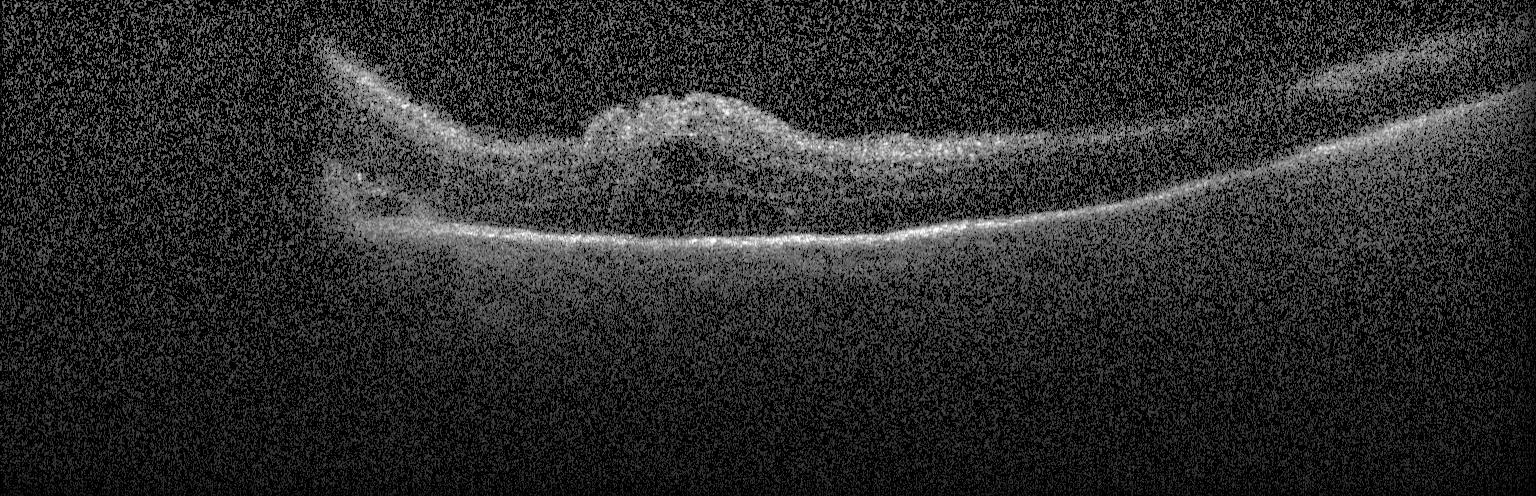 Spectral-domain OCT. Optical coherence tomography scan. Fovea-centered. Diabetic macular edema.